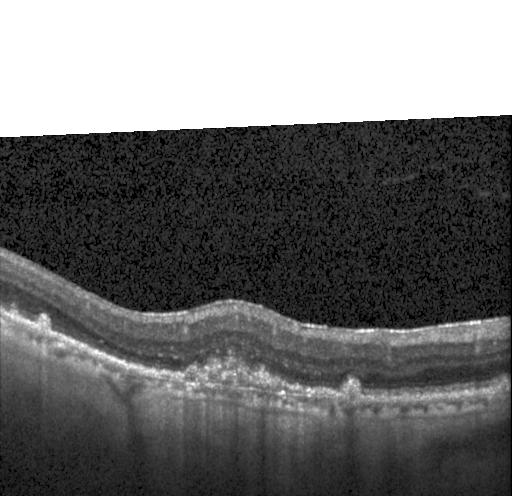
Retinal OCT cross-section showing choroidal neovascularization.